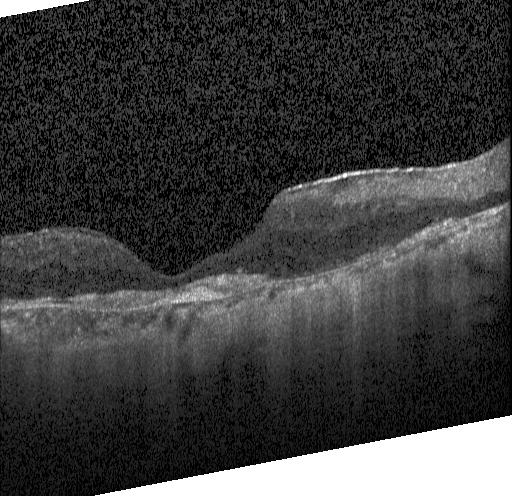
Heidelberg Spectralis, spectral-domain optical coherence tomography, retinal OCT cross-section
Finding: CNV.